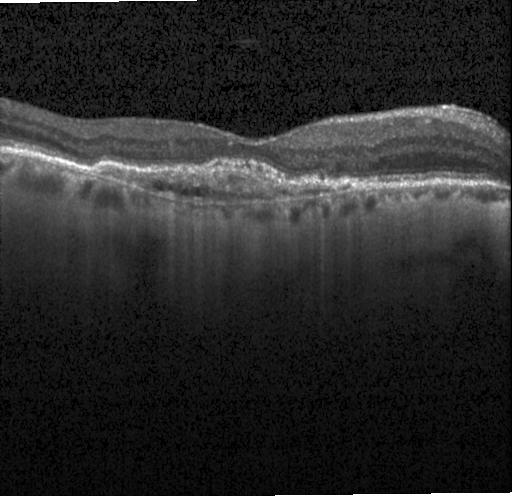
Heidelberg Spectralis · optical coherence tomography scan. The scan shows choroidal neovascularization (CNV).